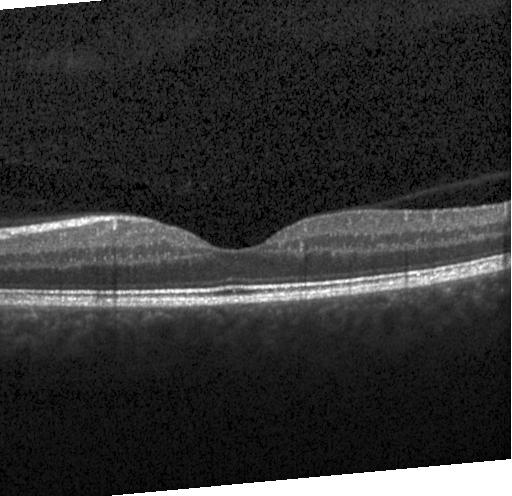
Retinal OCT B-scan, SD-OCT. Impression: no choroidal neovascularization, diabetic macular edema, or drusen.